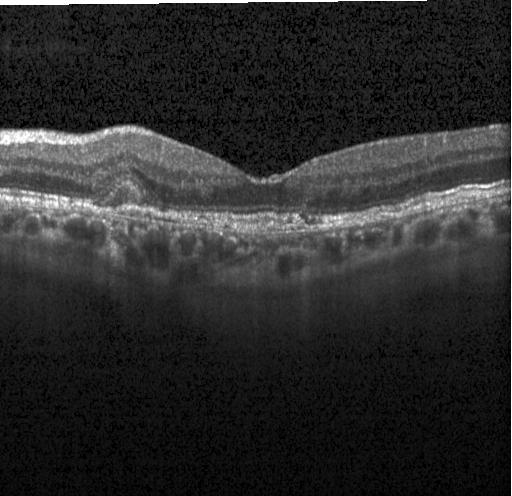 Fovea-centered. OCT B-scan. Instrument: Heidelberg Spectralis — Finding: sub-RPE drusenoid deposits.